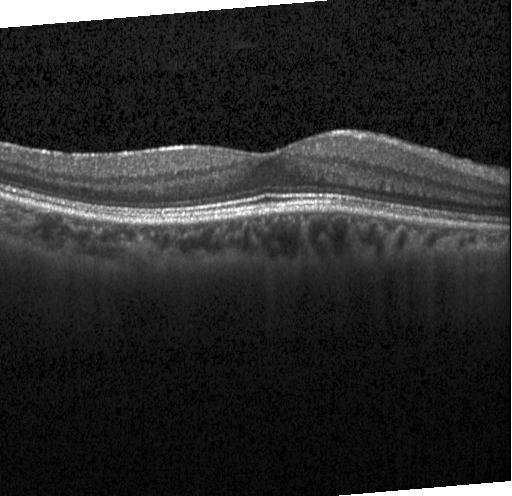
Retinal OCT cross-section showing neither choroidal neovascularization, diabetic macular edema, nor drusen.